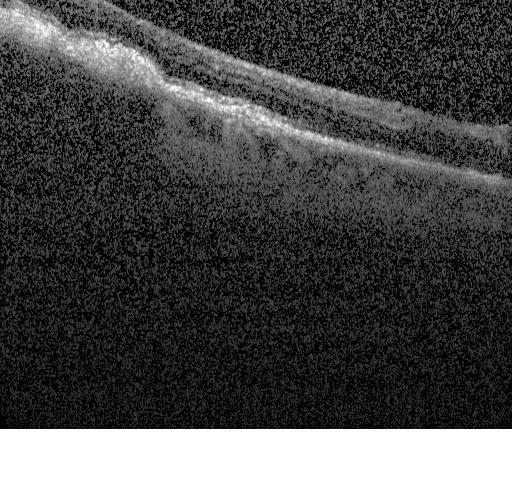
Acquired on a Heidelberg Spectralis; optical coherence tomography B-scan. Assessment: choroidal neovascularization (CNV).